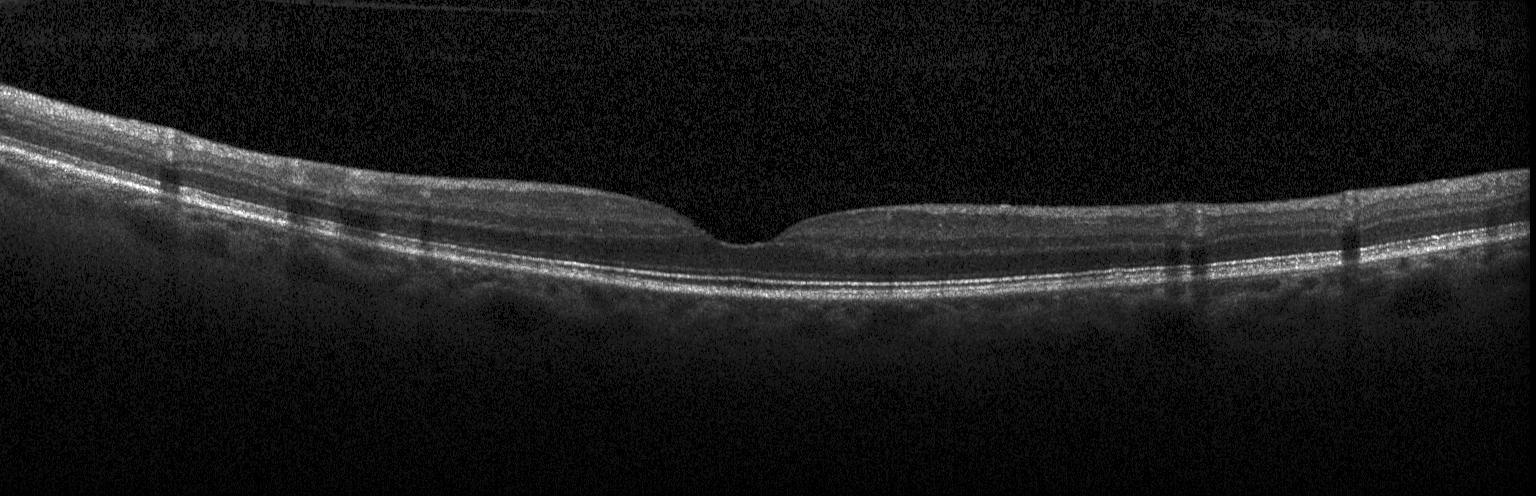
Diagnosis: neither CNV, DME, nor drusen.